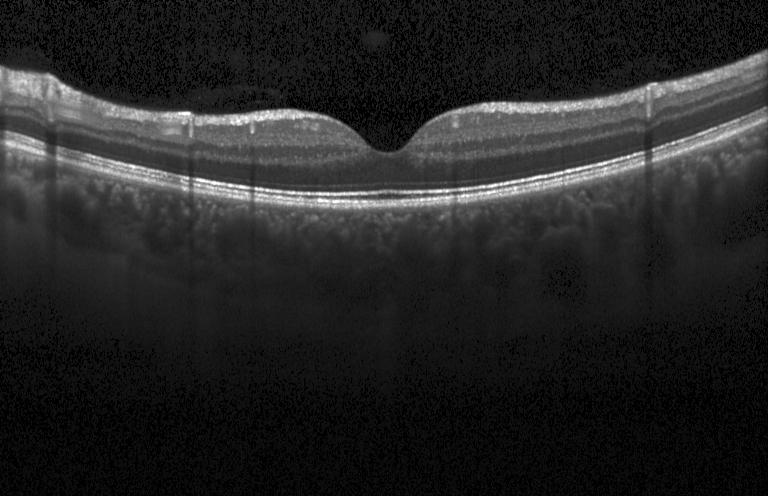
Impression: neither choroidal neovascularization, diabetic macular edema, nor drusen.